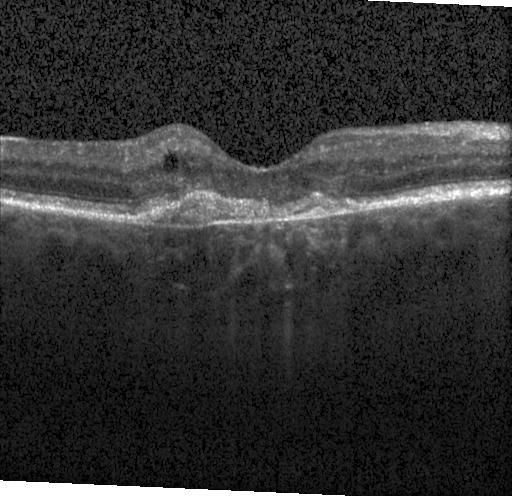 Retinal OCT B-scan — Diagnosis: CNV.